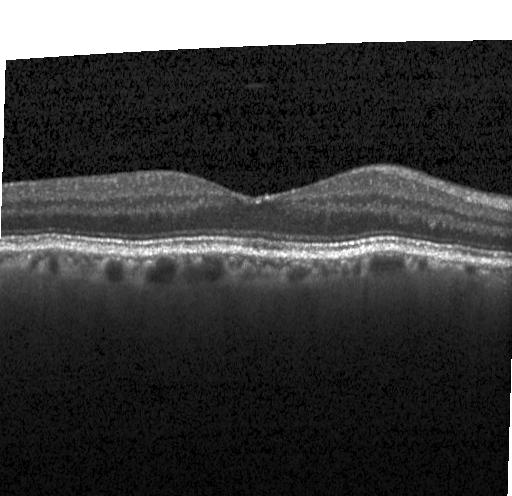 Spectral-domain OCT B-scan: no choroidal neovascularization, no diabetic macular edema, and no drusen.